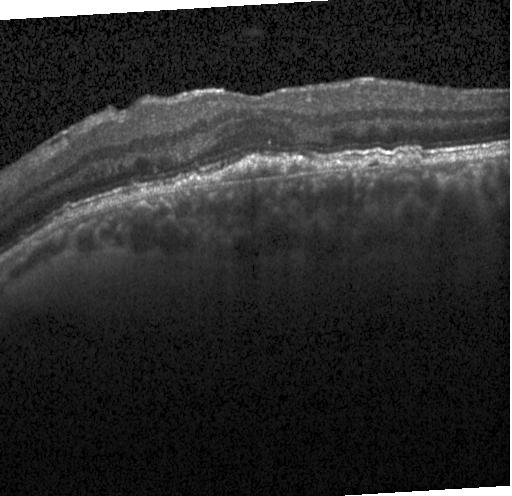 Retinal OCT cross-section
This B-scan demonstrates a choroidal neovascular membrane.